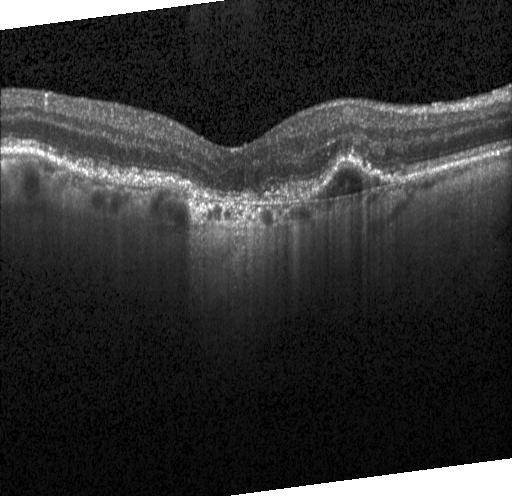

Heidelberg Spectralis OCT system. OCT line scan.
Assessment: a choroidal neovascular membrane.